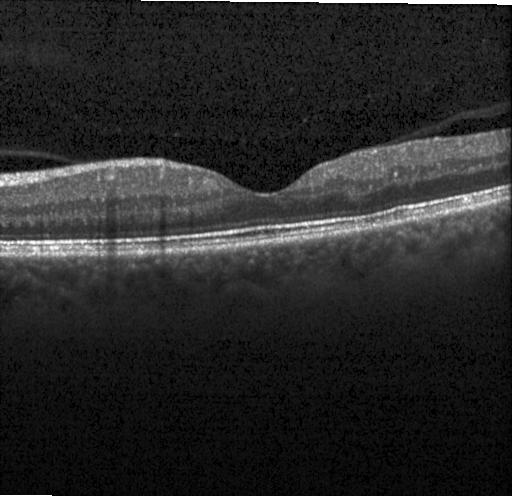 Optical coherence tomography B-scan · SD-OCT — This B-scan demonstrates no choroidal neovascularization, no diabetic macular edema, and no drusen.